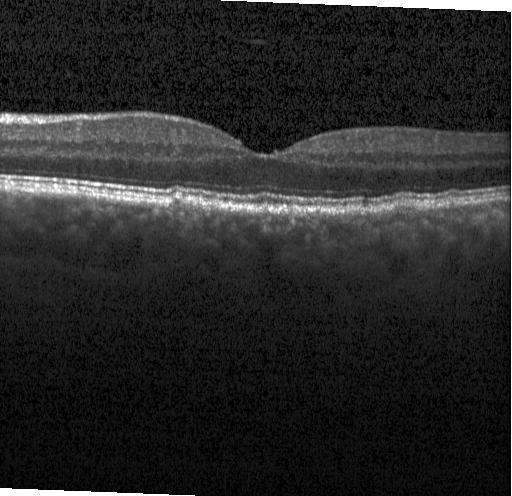

Impression: sub-RPE drusenoid deposits.